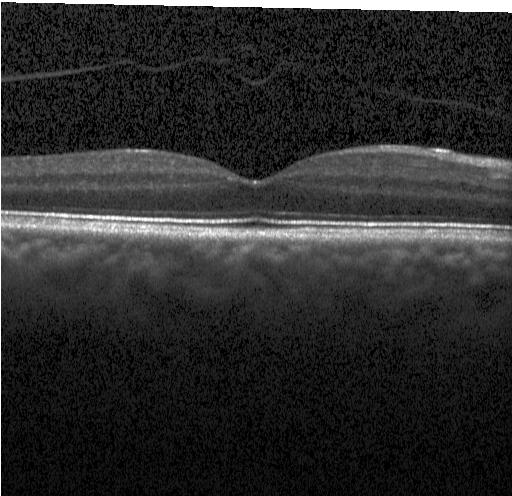 OCT B-scan showing neither choroidal neovascularization, diabetic macular edema, nor drusen.